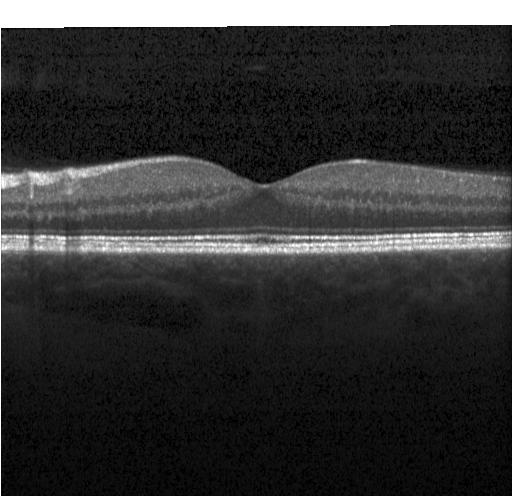 Neither choroidal neovascularization, diabetic macular edema, nor drusen.